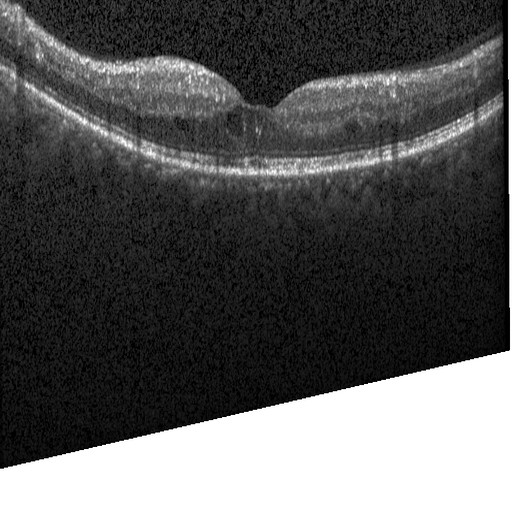

Retinal OCT B-scan. Spectral-domain OCT
Assessment: diabetic macular edema.